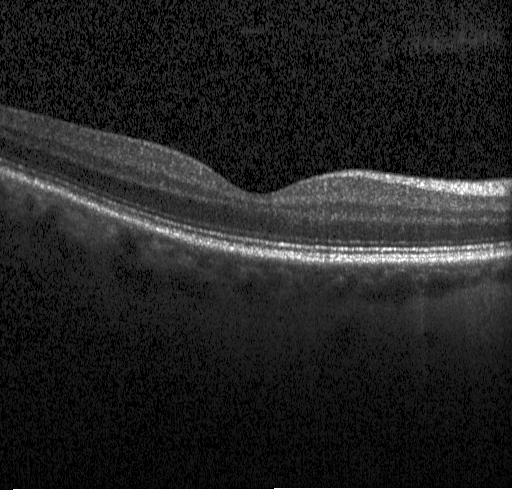
Dx: neither choroidal neovascularization, diabetic macular edema, nor drusen.